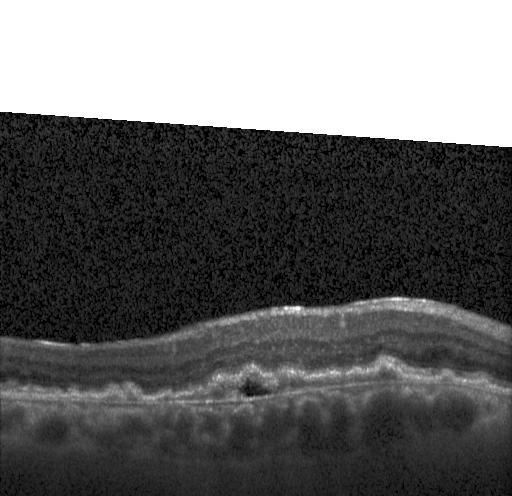

OCT finding: CNV.